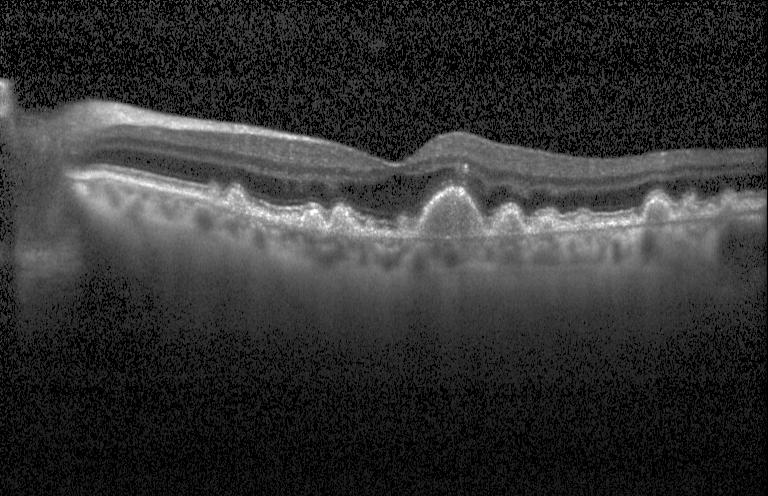
Retinal OCT cross-section
OCT finding: sub-RPE drusenoid deposits.